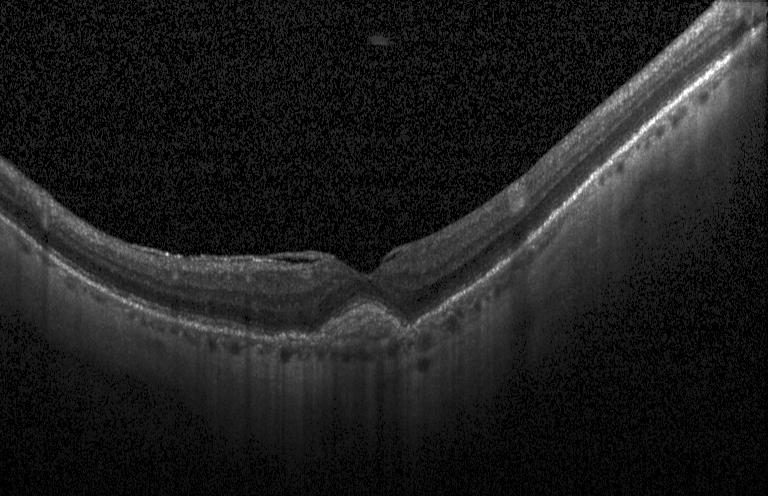 Diagnosis: a choroidal neovascular membrane.